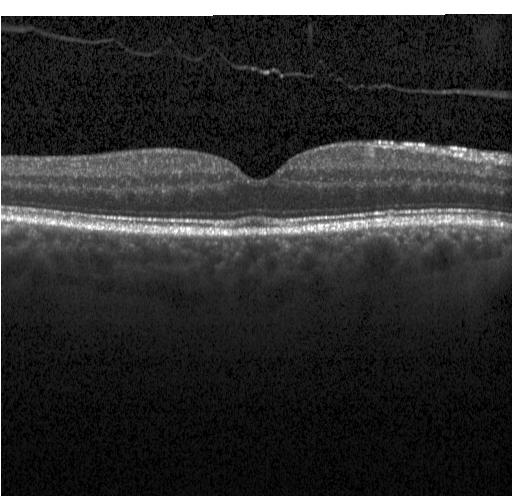

OCT finding: no evidence of choroidal neovascularization, diabetic macular edema, or drusen.